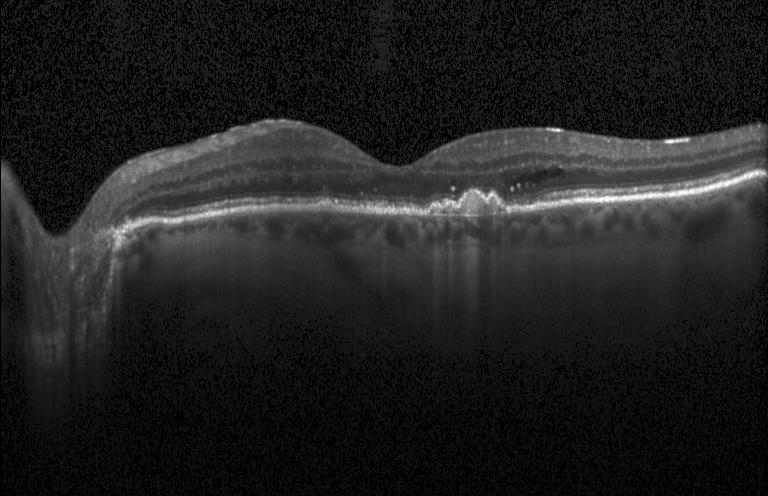 Macular OCT: sub-RPE drusenoid deposits.